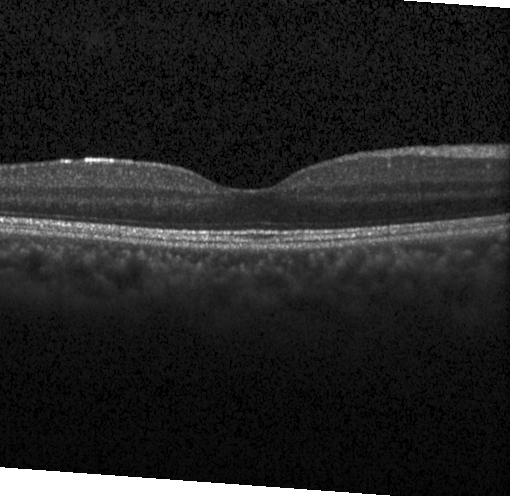
Macular scan, retinal OCT cross-section.
Dx: no evidence of choroidal neovascularization, diabetic macular edema, or drusen.